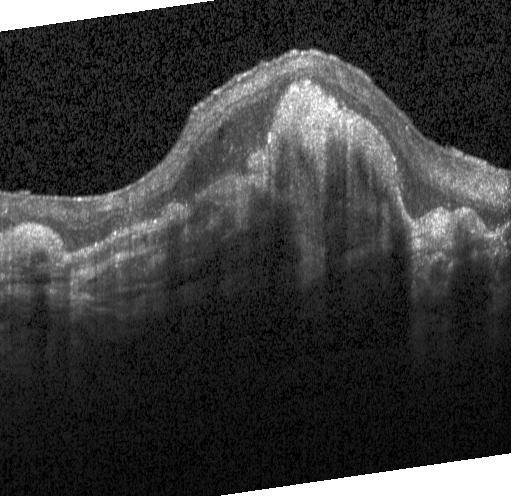

OCT line scan
A choroidal neovascular membrane.